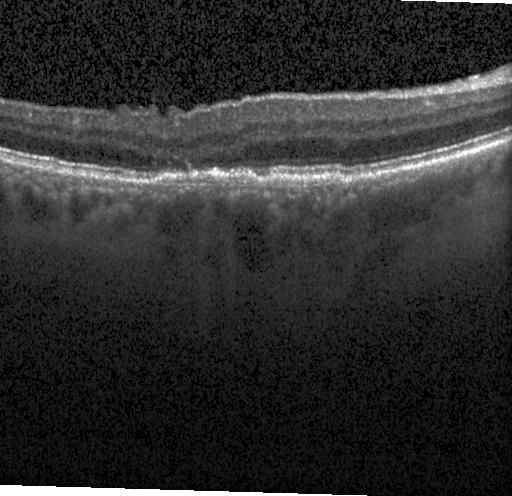
Optical coherence tomography B-scan — Finding: CNV.